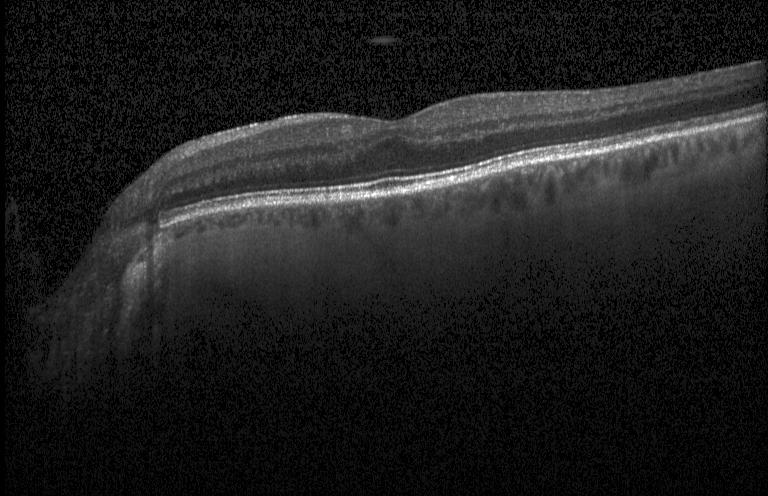

Finding: neither CNV, DME, nor drusen.